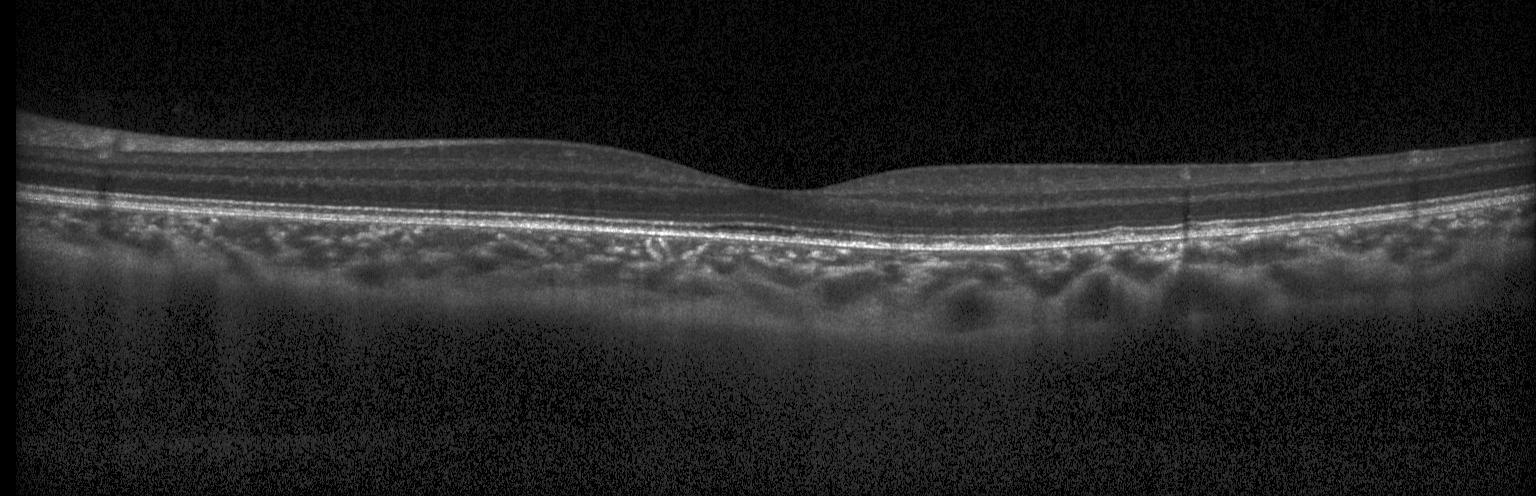
Retinal OCT cross-section
Neither choroidal neovascularization, diabetic macular edema, nor drusen.